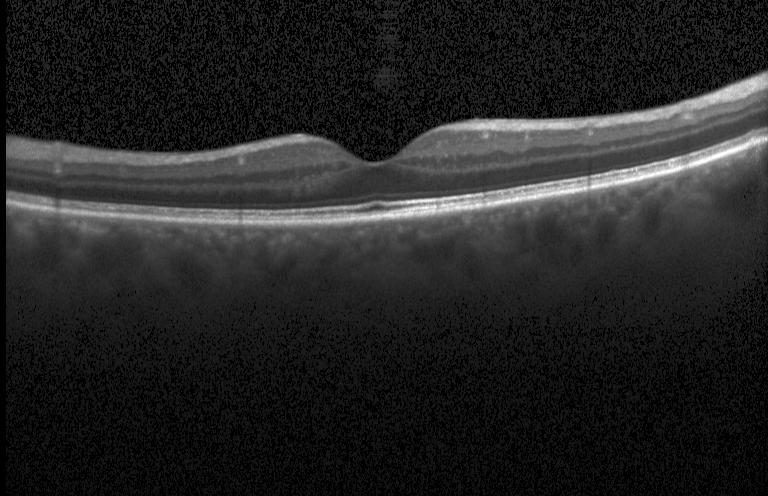
The scan shows no CNV, DME, or drusen.